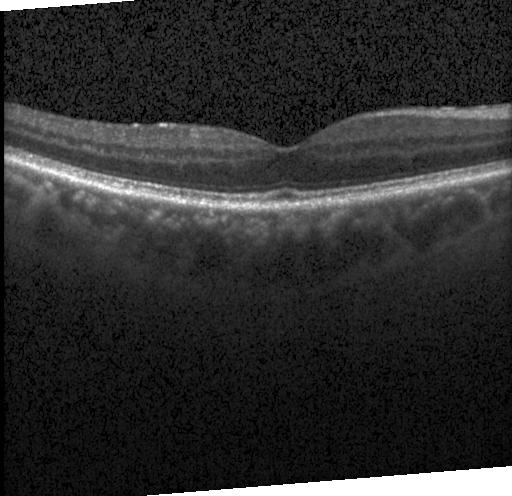
Dx: no CNV, DME, or drusen.